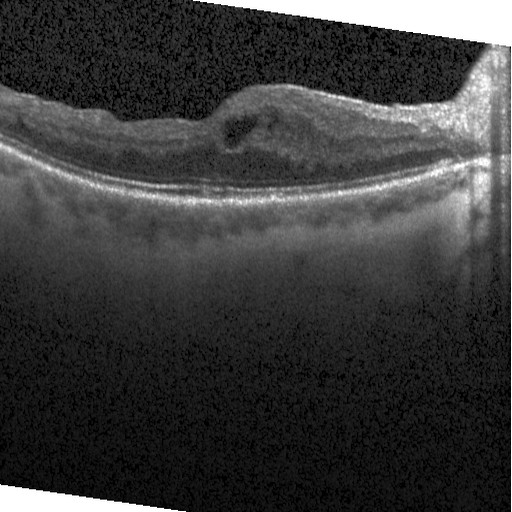 Retinal OCT B-scan.
Impression: diabetic macular edema (DME).